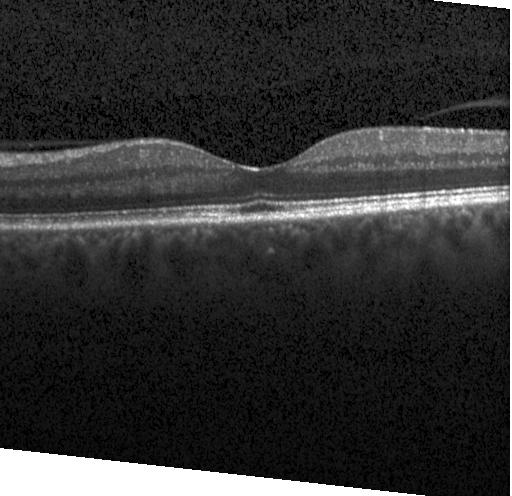

OCT scan showing neither choroidal neovascularization, diabetic macular edema, nor drusen.